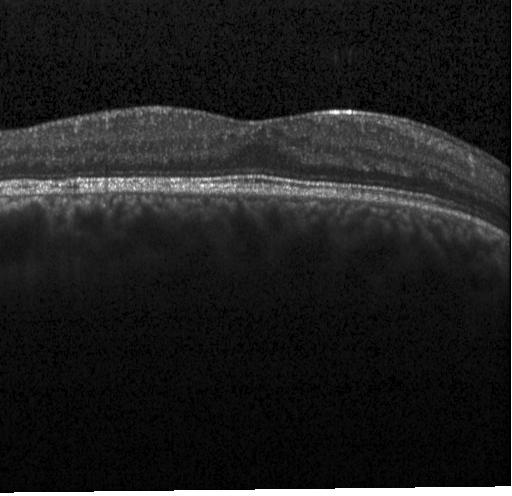 Finding: no choroidal neovascularization, diabetic macular edema, or drusen.